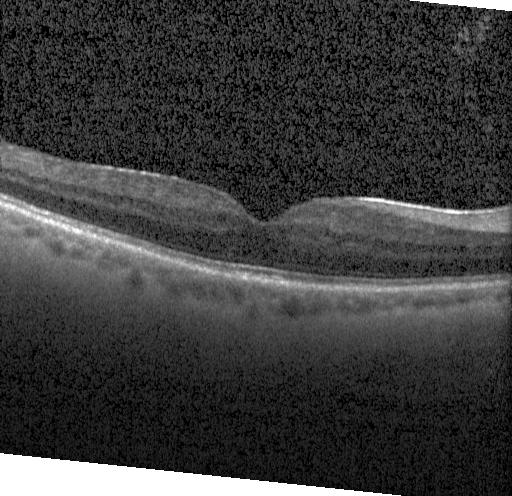
Optical coherence tomography B-scan, spectral-domain OCT.
This B-scan demonstrates no choroidal neovascularization, diabetic macular edema, or drusen.